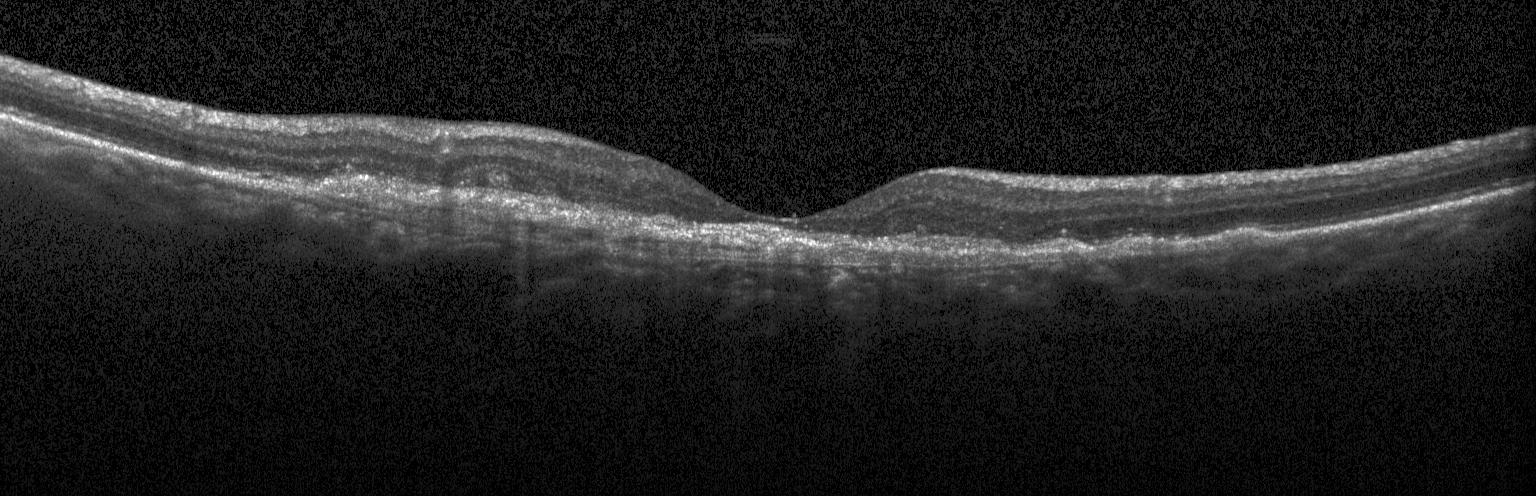
Diagnosis: choroidal neovascularization.